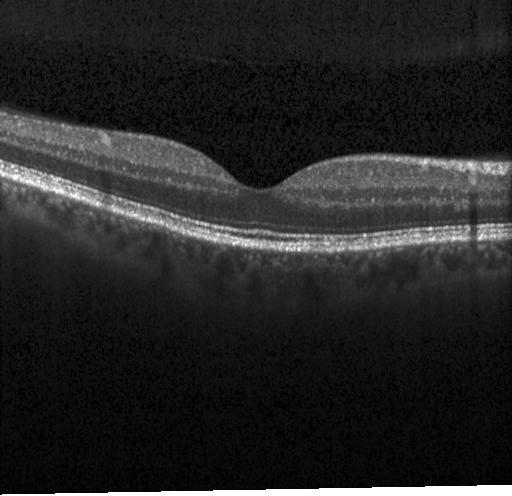

Optical coherence tomography scan.
No choroidal neovascularization, diabetic macular edema, or drusen.